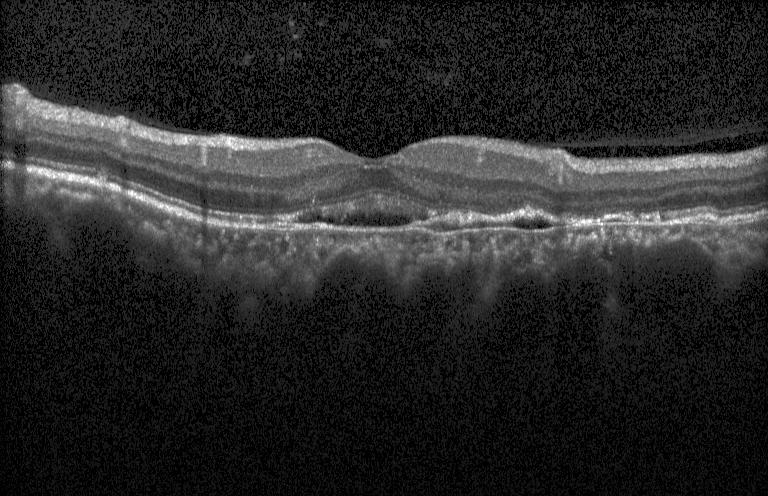 Optical coherence tomography B-scan, spectral-domain OCT.
Diagnosis: a choroidal neovascular membrane.